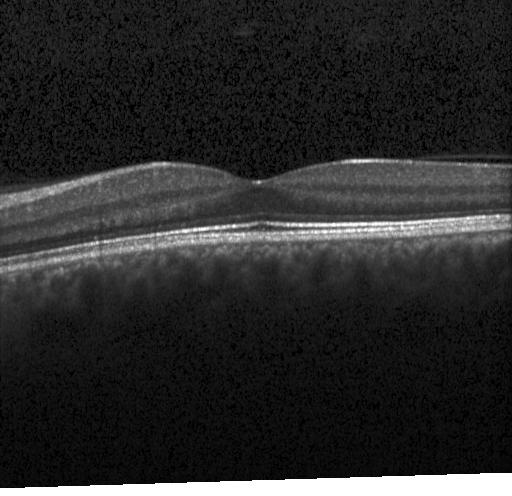 Assessment: no choroidal neovascularization, no diabetic macular edema, and no drusen.